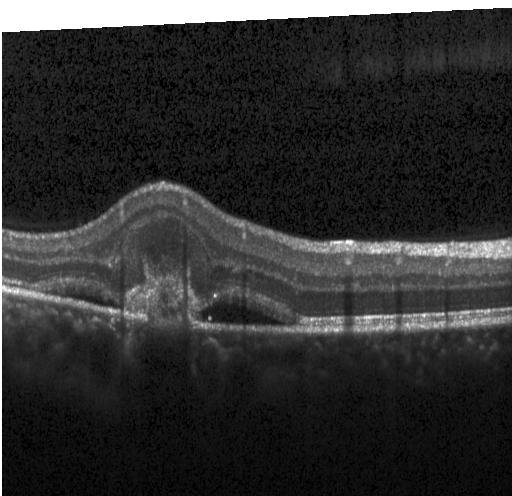
SD-OCT. Optical coherence tomography scan
Choroidal neovascularization.